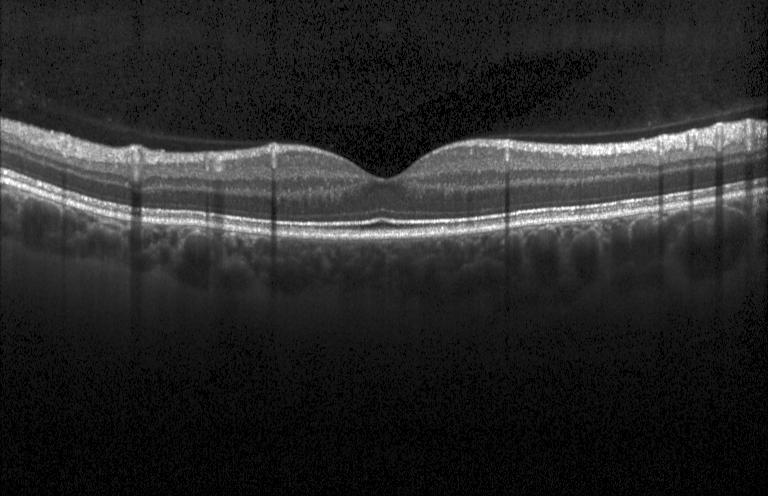 OCT B-scan showing no choroidal neovascularization, no diabetic macular edema, and no drusen.